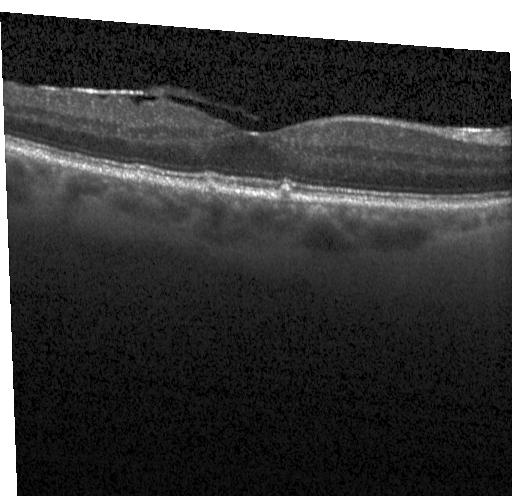

Multiple drusen.